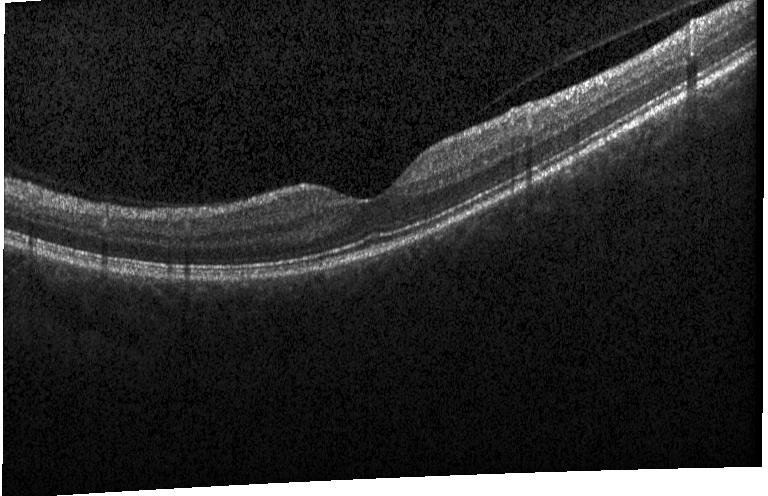
OCT B-scan.
The scan shows neither choroidal neovascularization, diabetic macular edema, nor drusen.